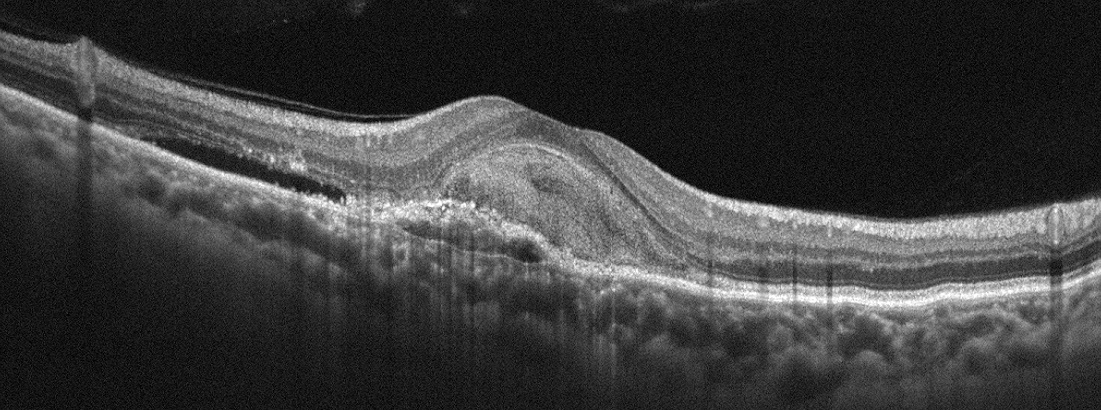
Macular OCT demonstrating AMD.